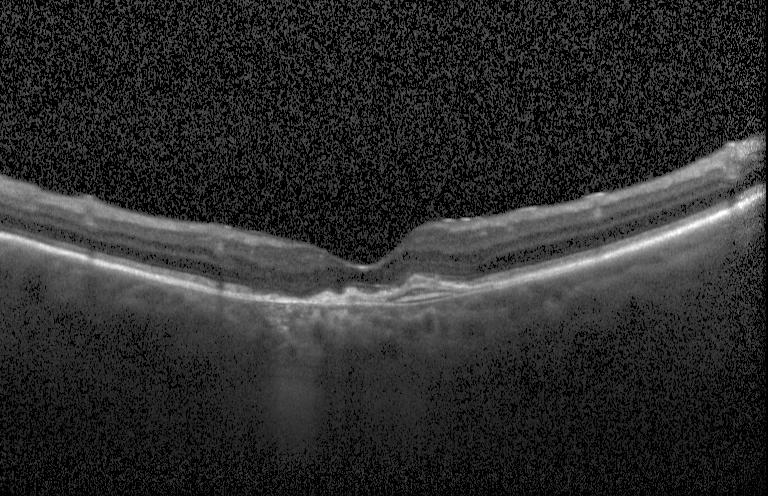
Impression: choroidal neovascularization (CNV).